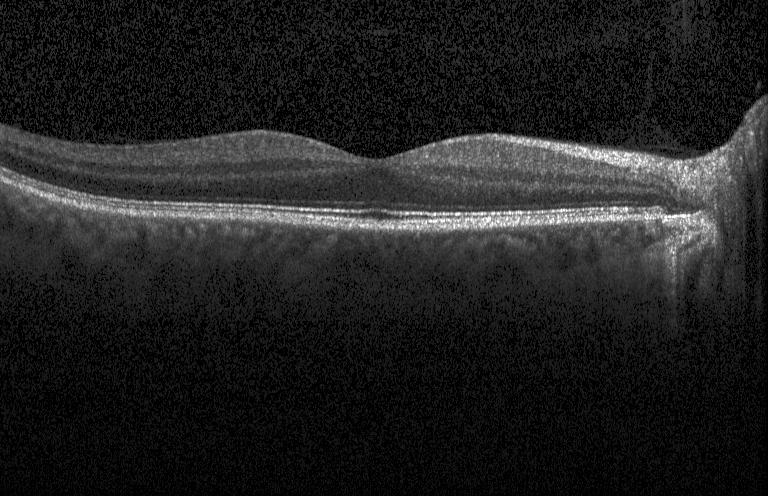 Retinal OCT cross-section.
Impression: no choroidal neovascularization, no diabetic macular edema, and no drusen.